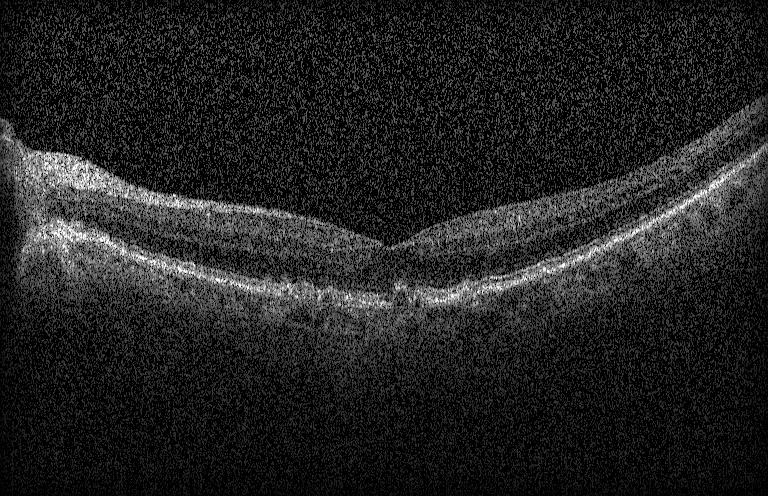
OCT B-scan; centered on the fovea
Finding: CNV.